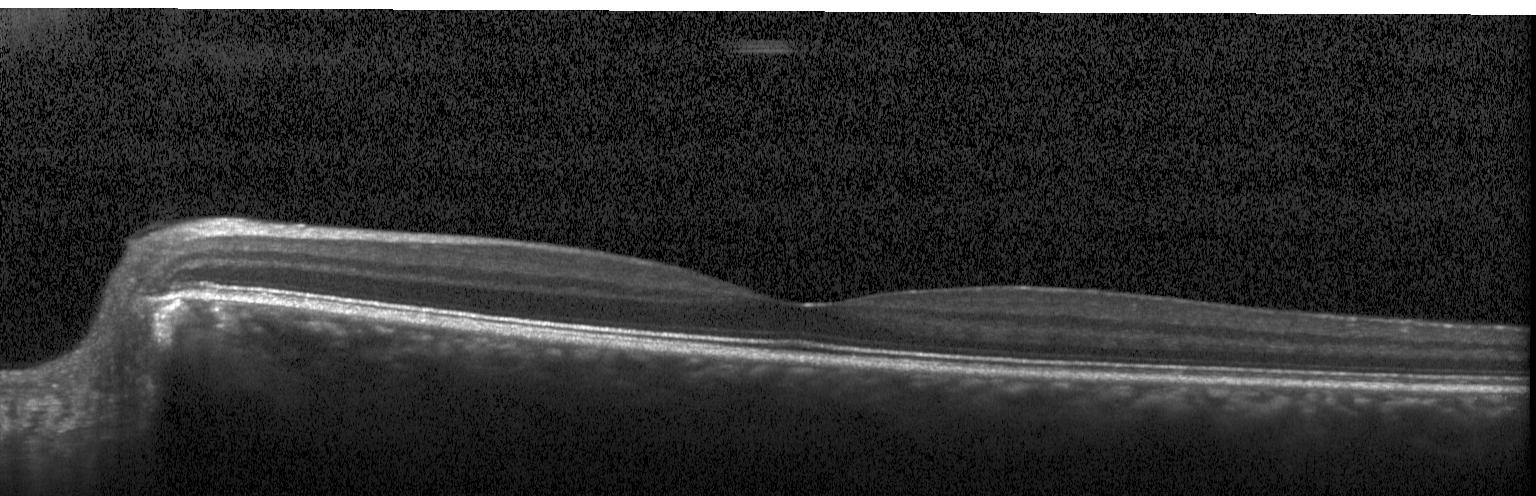

Impression: no CNV, DME, or drusen.